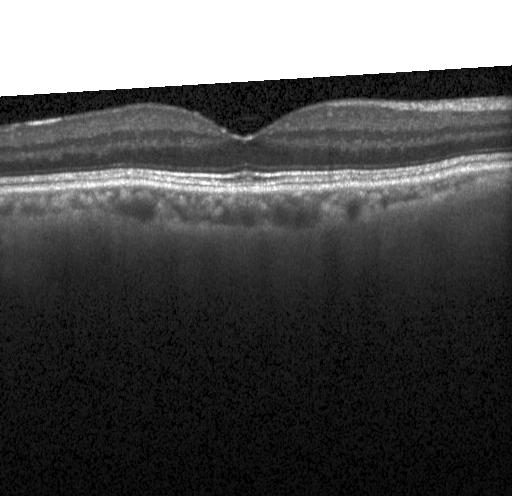

OCT B-scan showing no choroidal neovascularization, diabetic macular edema, or drusen.